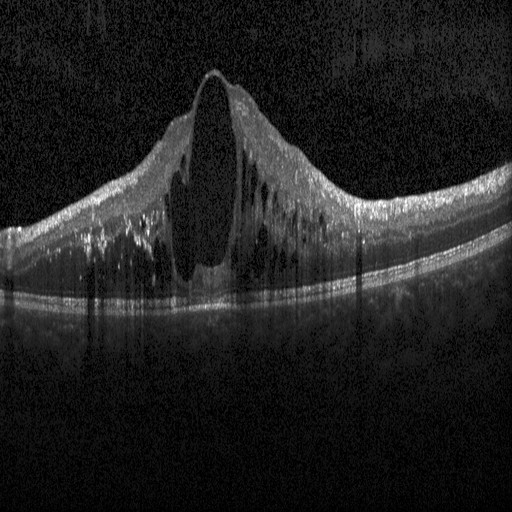
Impression: DME.